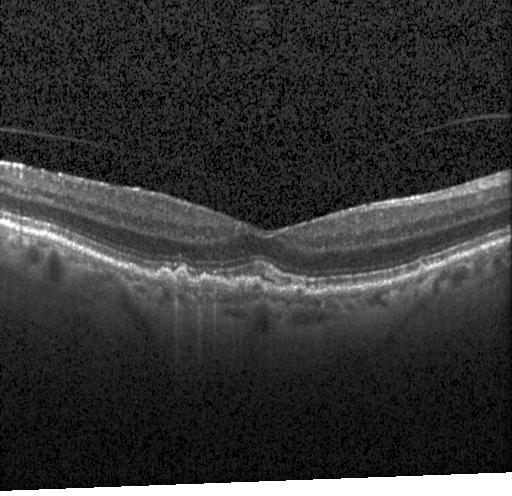 Impression: CNV.